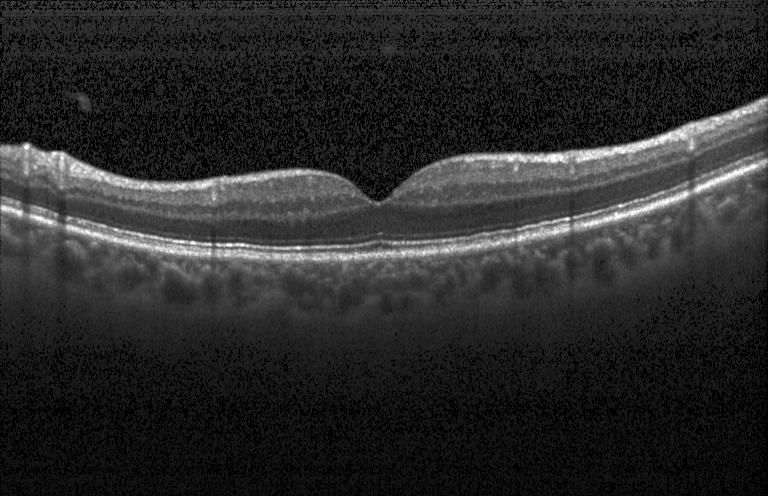
Diagnosis: neither choroidal neovascularization, diabetic macular edema, nor drusen.